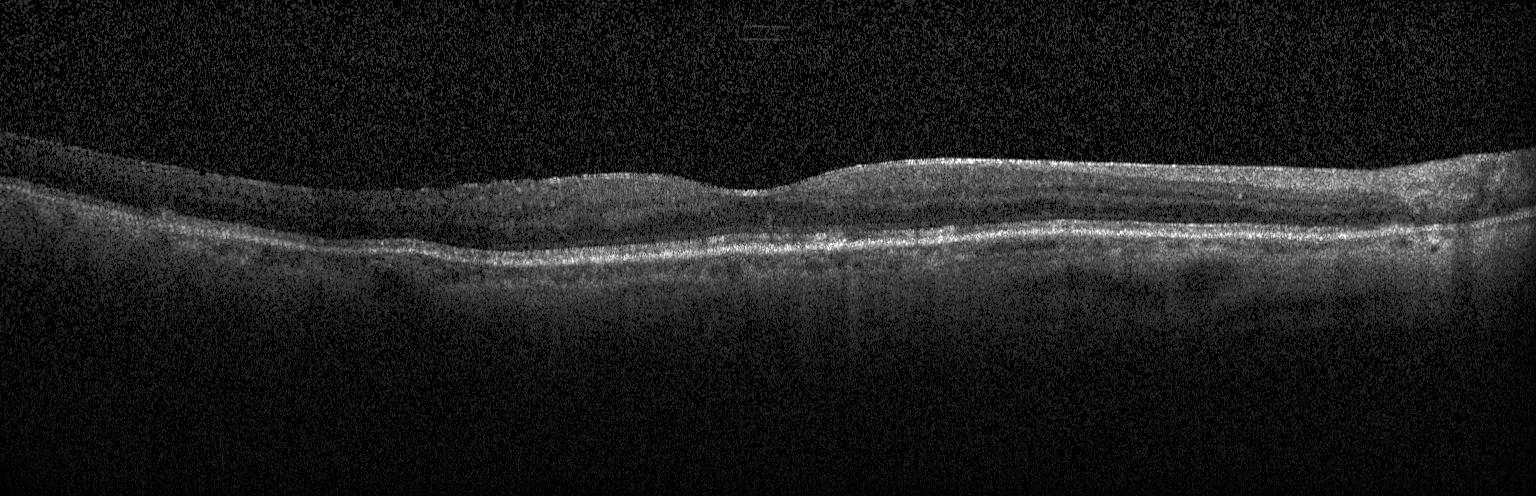

SD-OCT · acquired on a Heidelberg Spectralis · OCT line scan · centered on the fovea. Macular OCT: no CNV, no DME, and no drusen.